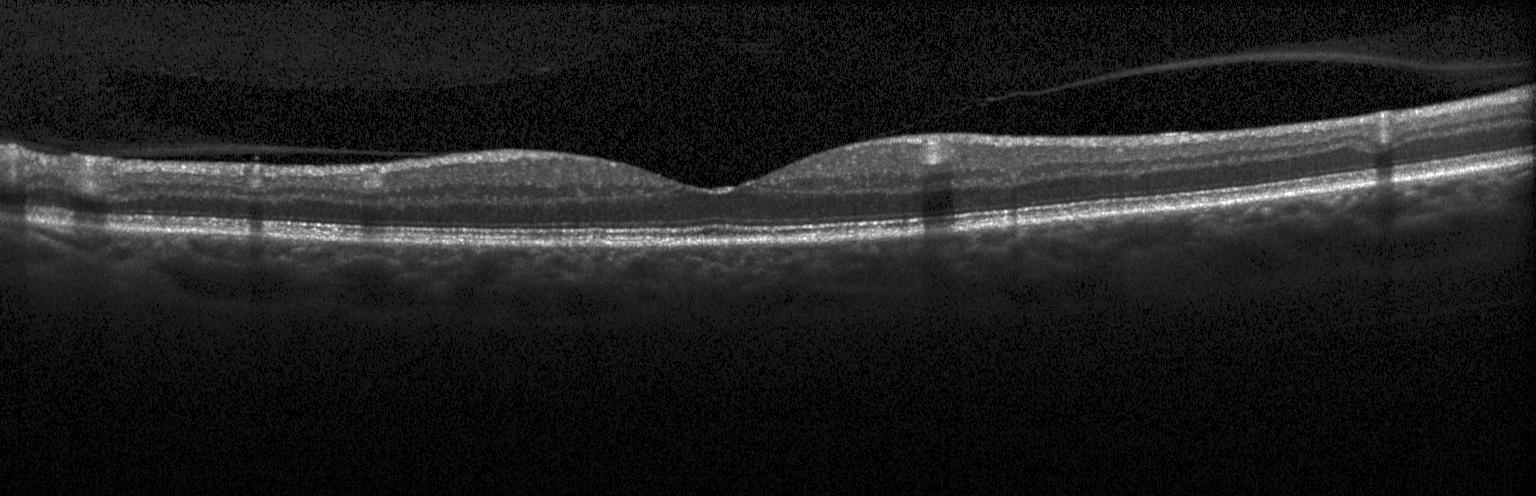 Macular OCT: no evidence of CNV, DME, or drusen.